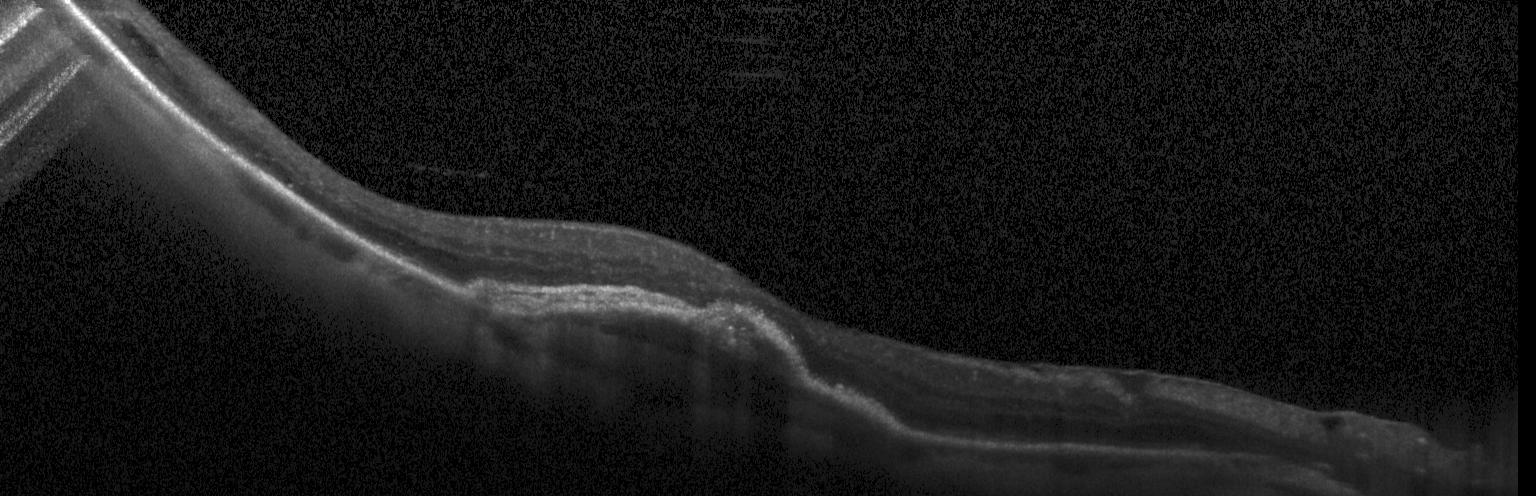
Centered on the fovea · SD-OCT · optical coherence tomography B-scan — Diagnosis: choroidal neovascularization.